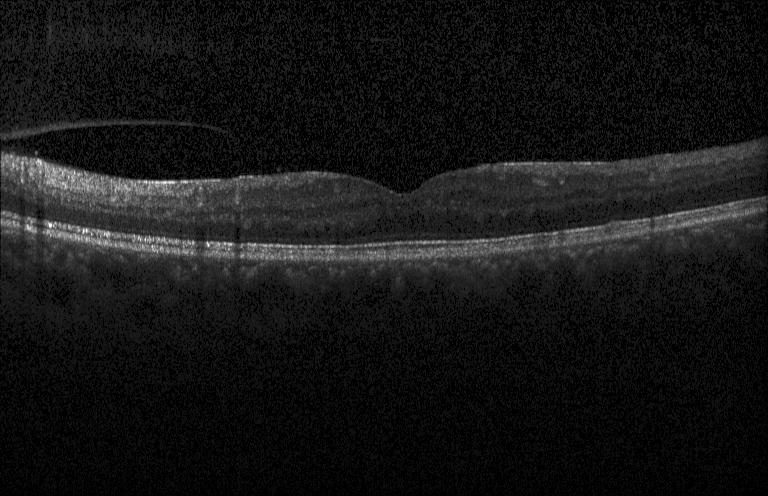

Dx: no choroidal neovascularization, diabetic macular edema, or drusen.